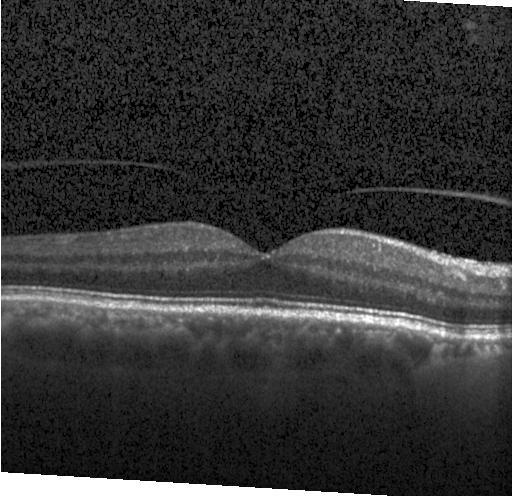
Acquired on a Heidelberg Spectralis · spectral-domain OCT · OCT line scan
Dx: no choroidal neovascularization, no diabetic macular edema, and no drusen.